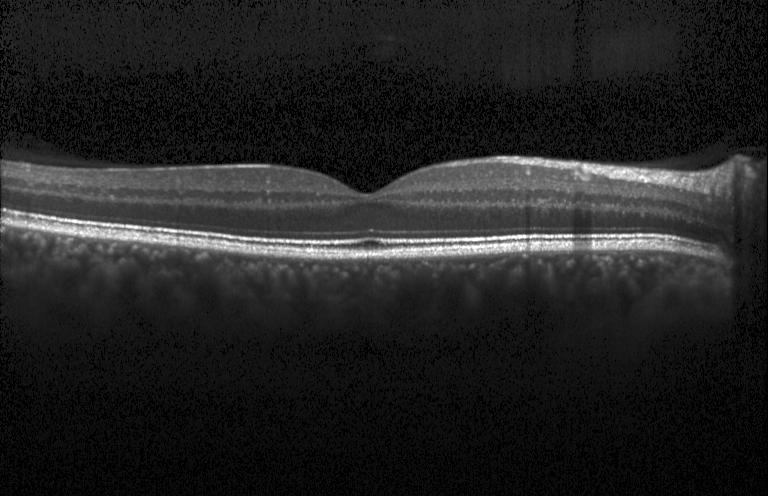

Optical coherence tomography scan · spectral-domain optical coherence tomography · Heidelberg Spectralis OCT system · fovea-centered — The scan shows no choroidal neovascularization, no diabetic macular edema, and no drusen.